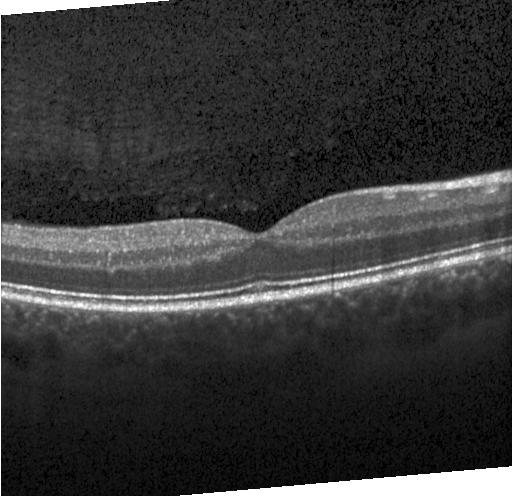 Macular scan. Optical coherence tomography B-scan. Dx: neither choroidal neovascularization, diabetic macular edema, nor drusen.